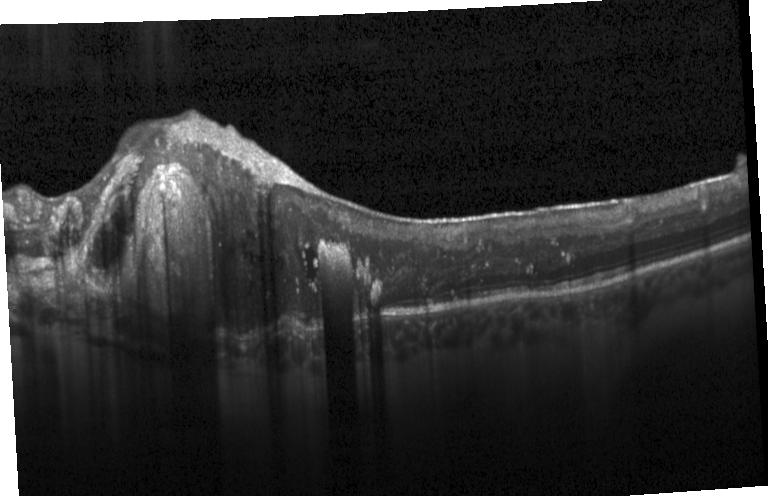

Optical coherence tomography scan
Macular OCT: a choroidal neovascular membrane.